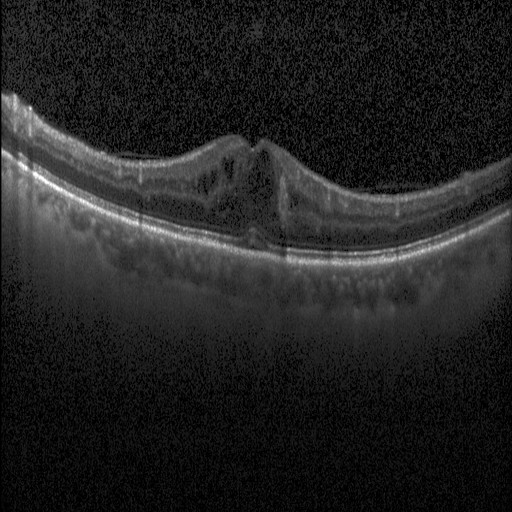 Through the macula, instrument: Heidelberg Spectralis, optical coherence tomography B-scan
Finding: DME.